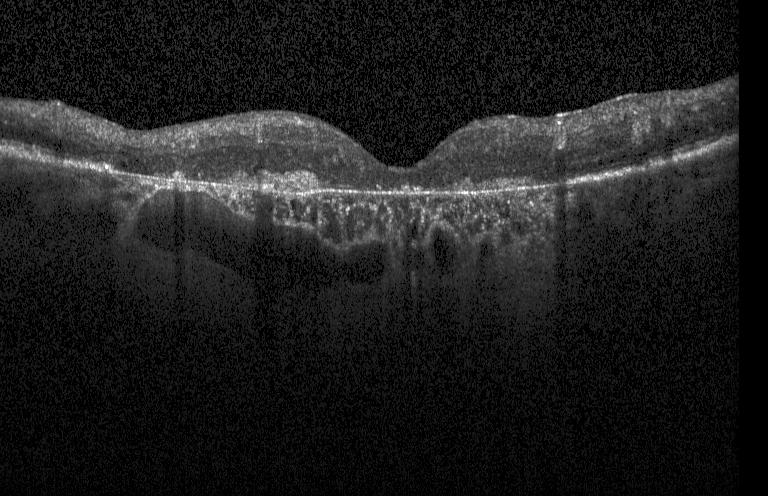 Optical coherence tomography scan
Assessment: choroidal neovascularization.